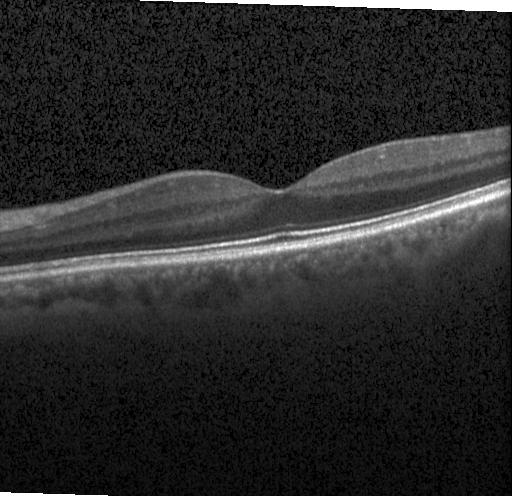
OCT line scan.
Finding: no choroidal neovascularization, diabetic macular edema, or drusen.